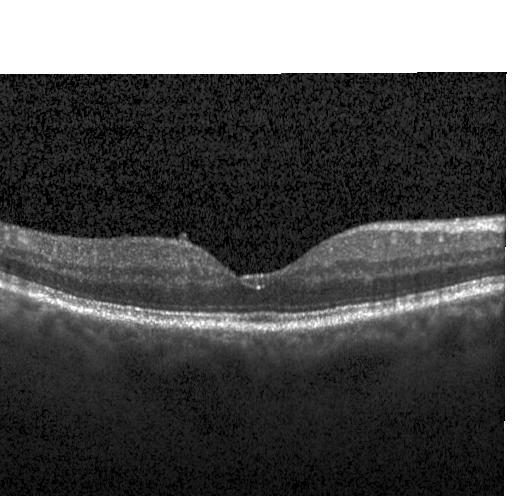 Retinal OCT cross-section showing no choroidal neovascularization, diabetic macular edema, or drusen.